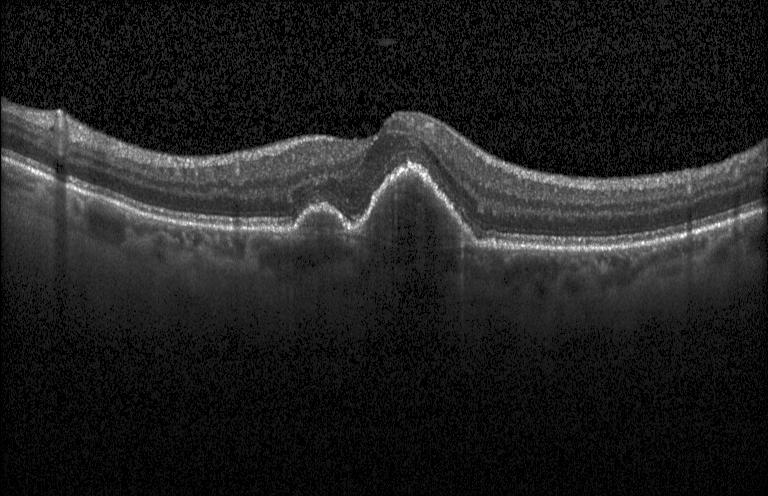

A choroidal neovascular membrane.